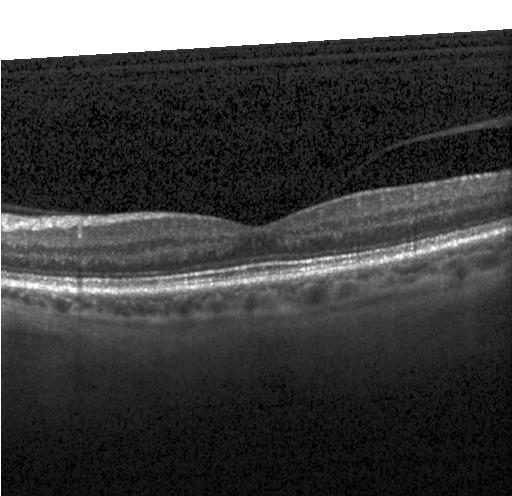
Retinal OCT B-scan. This B-scan demonstrates no choroidal neovascularization, no diabetic macular edema, and no drusen.